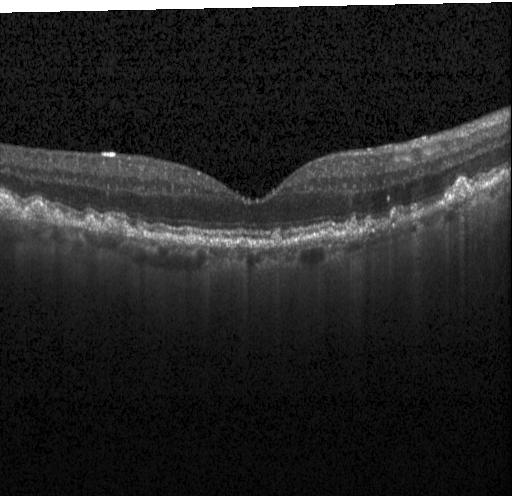 Retinal OCT B-scan — Diagnosis: sub-RPE drusenoid deposits.